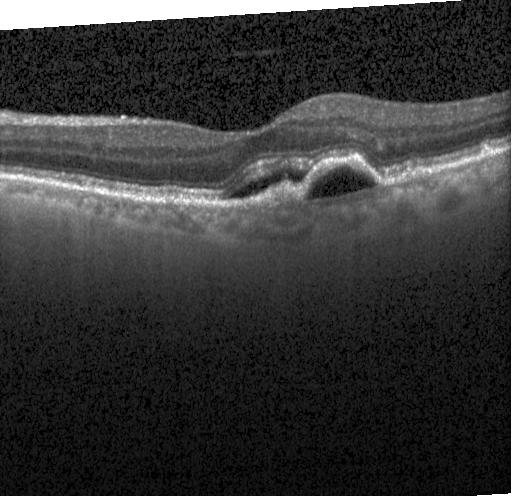 Impression: choroidal neovascularization (CNV).